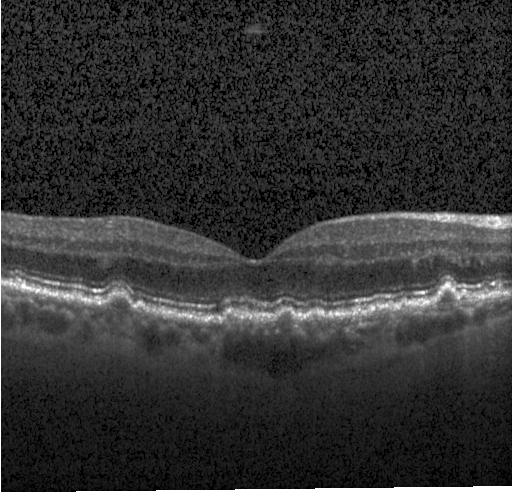 Diagnosis: sub-RPE drusenoid deposits.